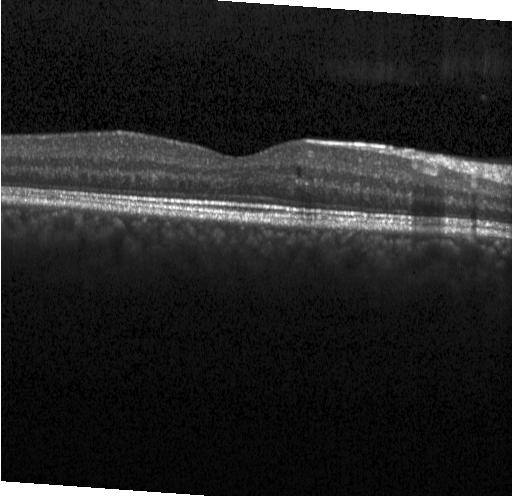
Optical coherence tomography B-scan. Diagnosis: diabetic macular edema.